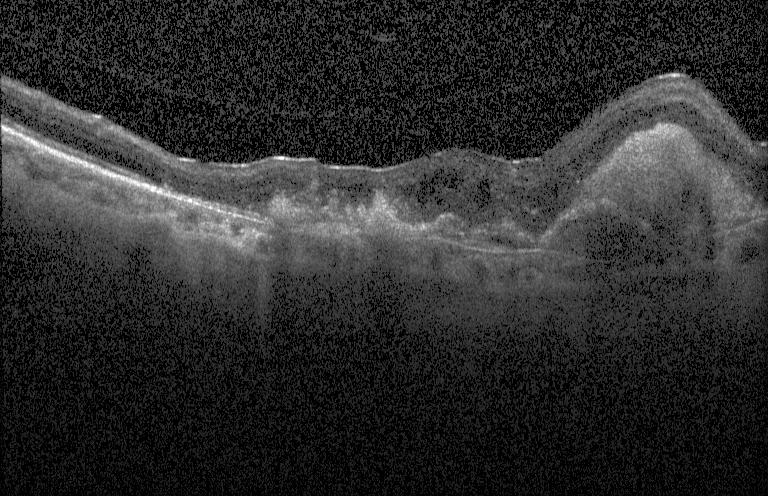 Retinal OCT cross-section. Impression: a choroidal neovascular membrane.